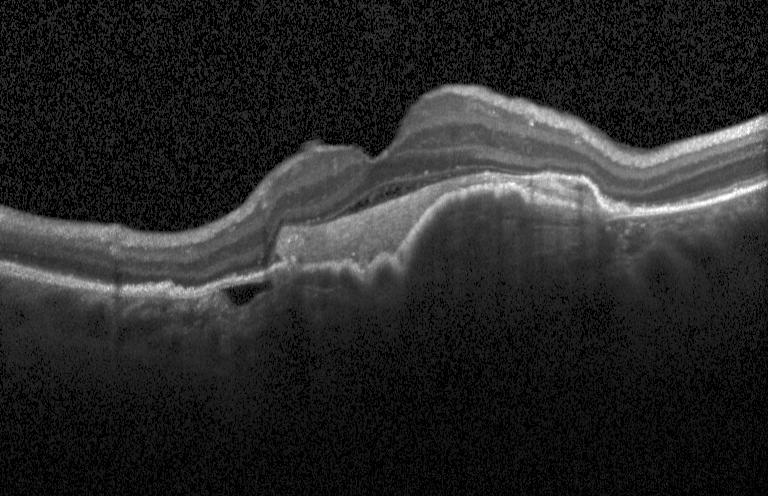
OCT B-scan · instrument: Heidelberg Spectralis · spectral-domain optical coherence tomography · macular scan. Diagnosis: a choroidal neovascular membrane.